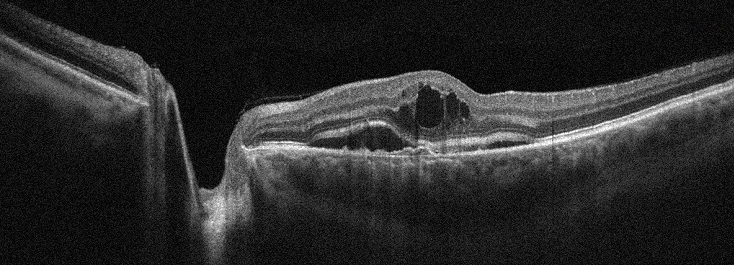

OCT B-scan. Macular OCT: age-related macular degeneration (AMD).